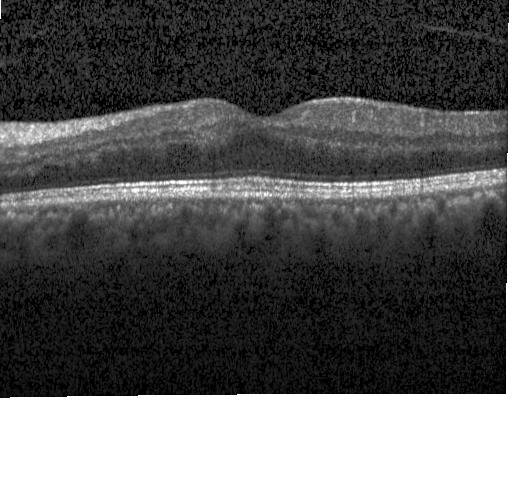 Impression: no evidence of choroidal neovascularization, diabetic macular edema, or drusen.